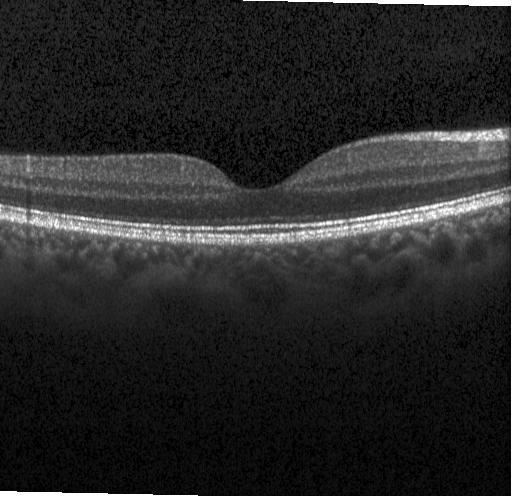
Retinal OCT cross-section — This B-scan demonstrates no CNV, DME, or drusen.